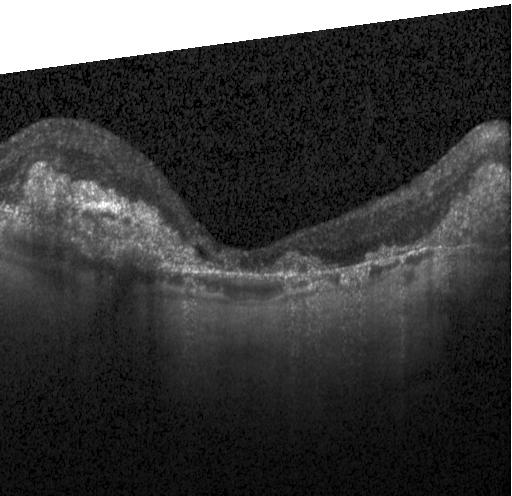

Horizontal scan through the fovea, optical coherence tomography B-scan, acquired on a Heidelberg Spectralis, spectral-domain optical coherence tomography — The scan shows CNV.